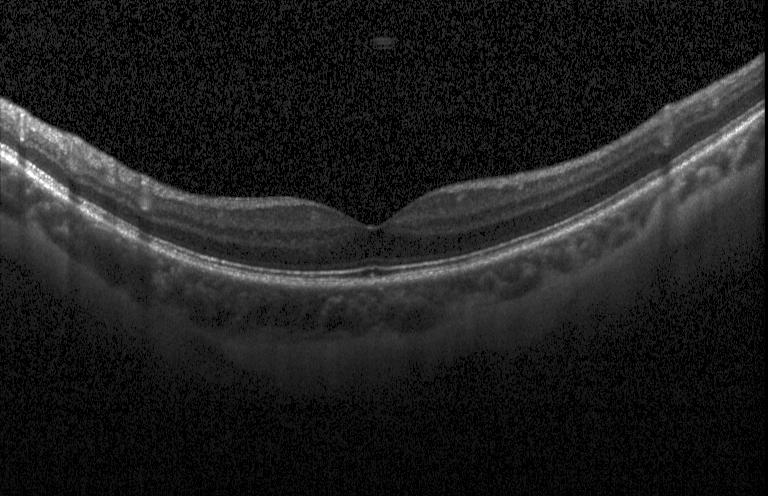 Finding: no choroidal neovascularization, diabetic macular edema, or drusen.